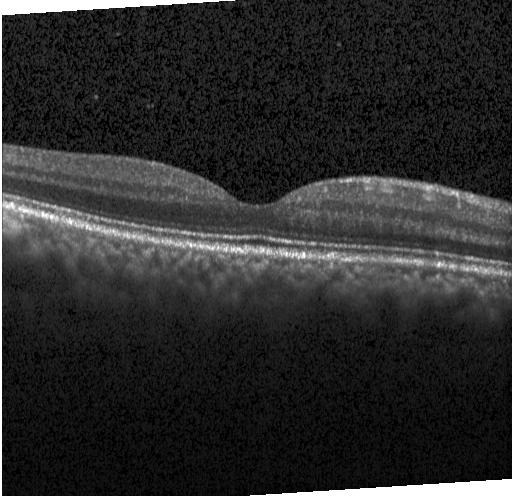
Retinal OCT B-scan. Assessment: no choroidal neovascularization, diabetic macular edema, or drusen.